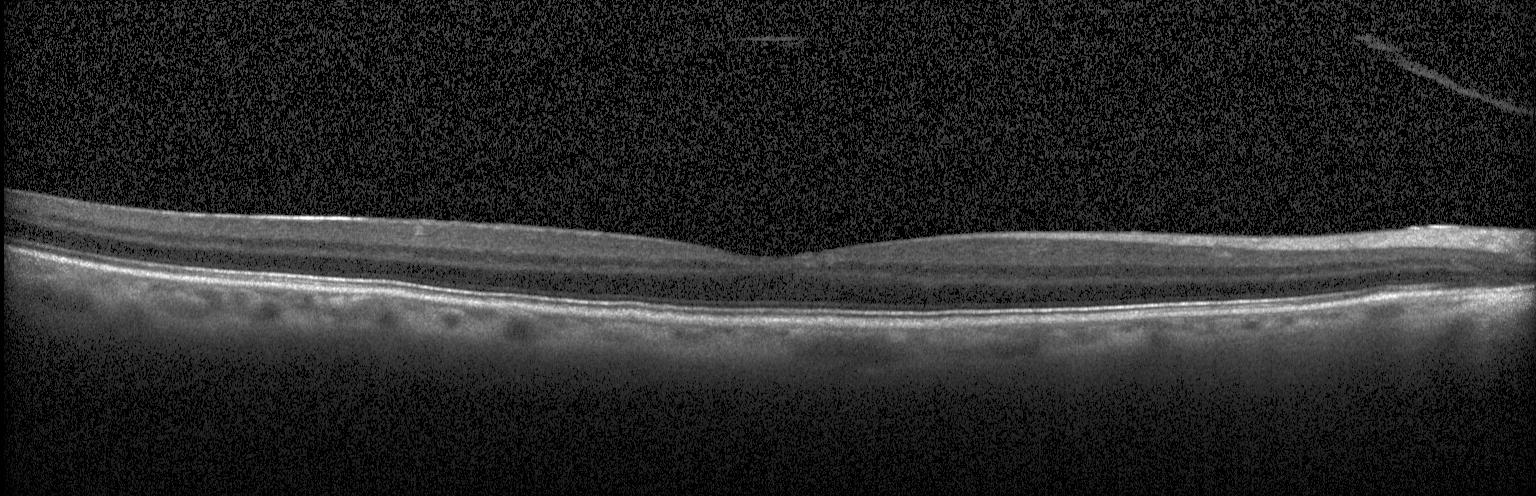 The scan shows no CNV, no DME, and no drusen.